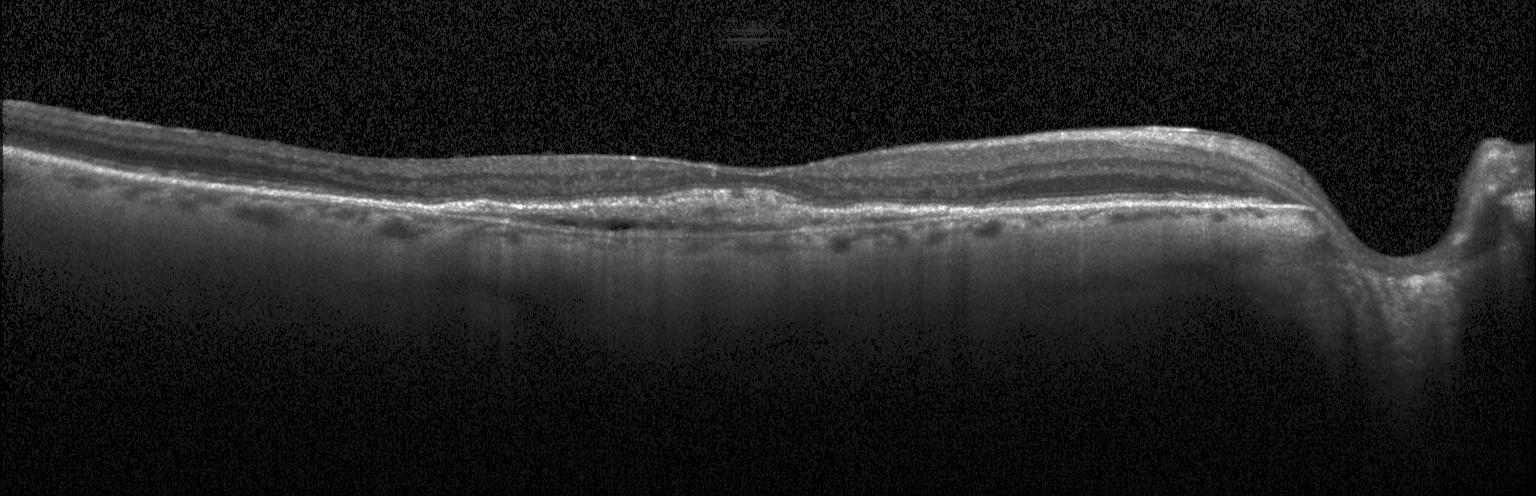
OCT line scan, acquired on a Heidelberg Spectralis, macular scan
OCT finding: a choroidal neovascular membrane.